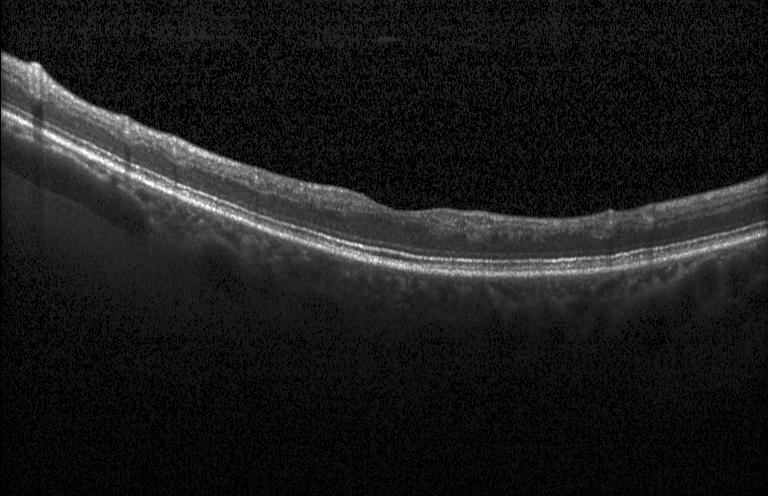

Optical coherence tomography scan · instrument: Heidelberg Spectralis — The scan shows no CNV, DME, or drusen.